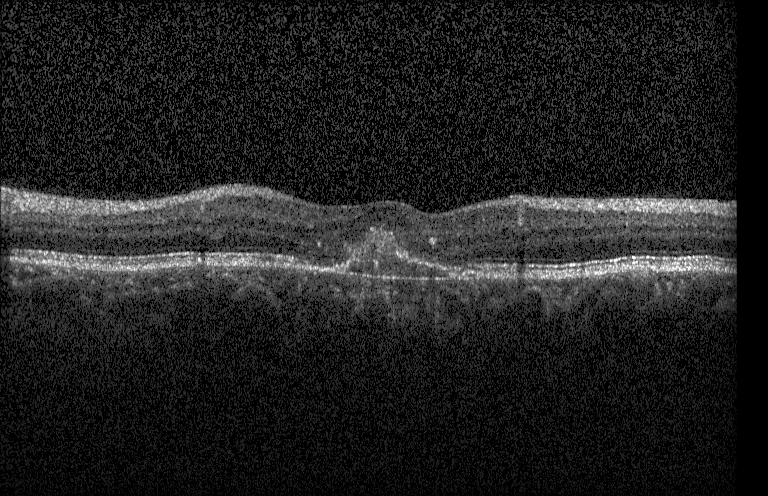 Finding: choroidal neovascularization.